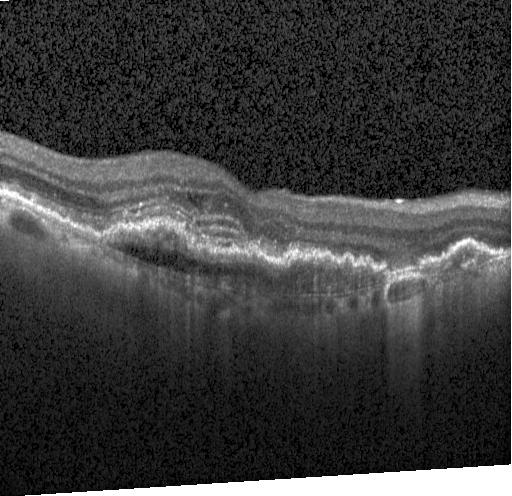 Optical coherence tomography scan — Dx: choroidal neovascularization (CNV).